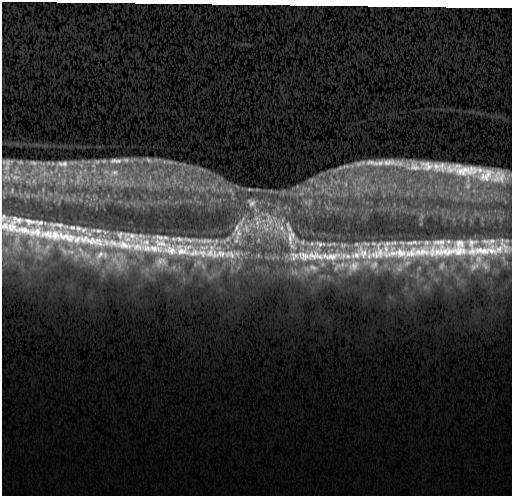

OCT B-scan. Heidelberg Spectralis OCT system.
Impression: a choroidal neovascular membrane.